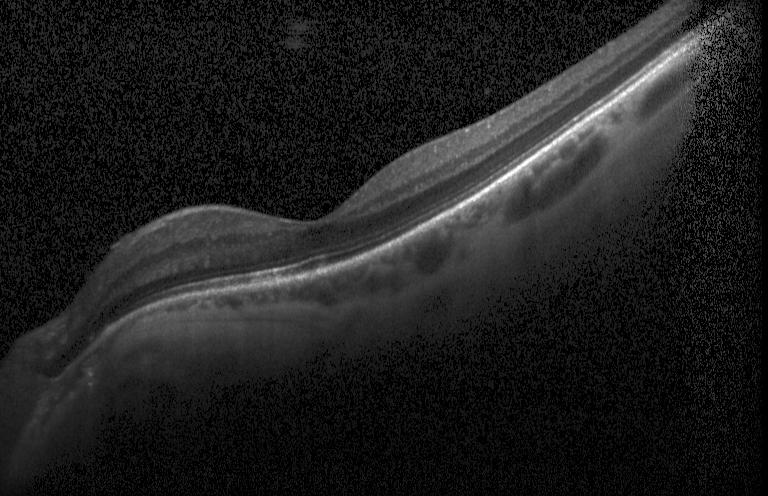 The scan shows neither CNV, DME, nor drusen.